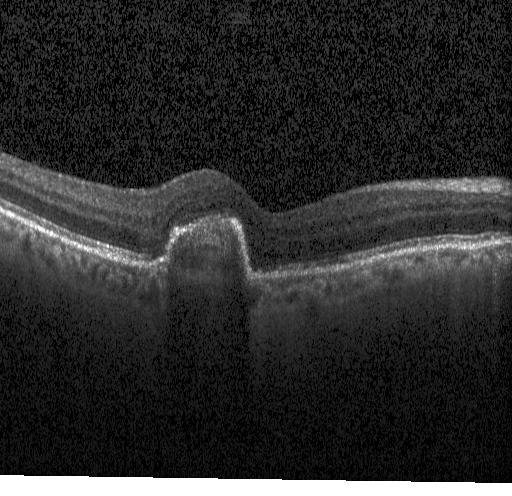

OCT scan showing choroidal neovascularization.